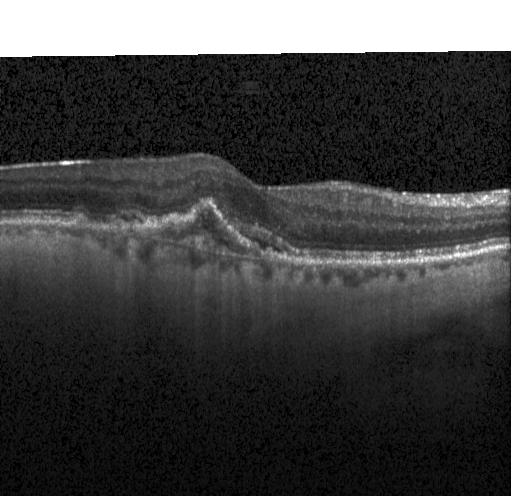
OCT B-scan · centered on the fovea.
Finding: CNV.